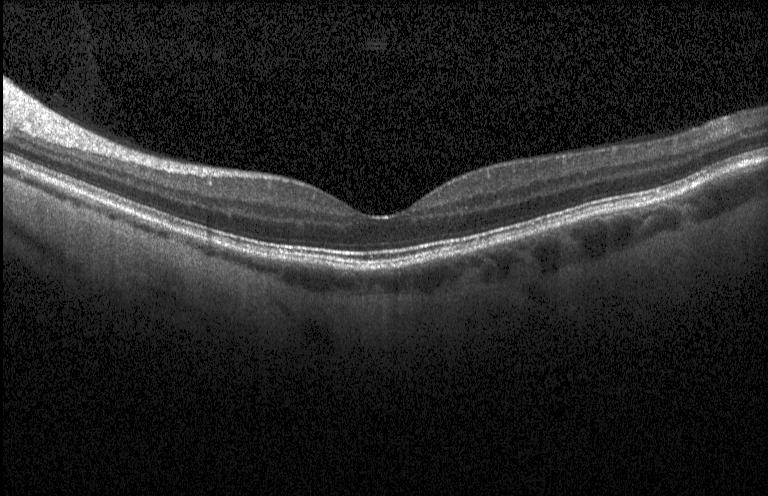 Retinal OCT B-scan. Dx: neither choroidal neovascularization, diabetic macular edema, nor drusen.